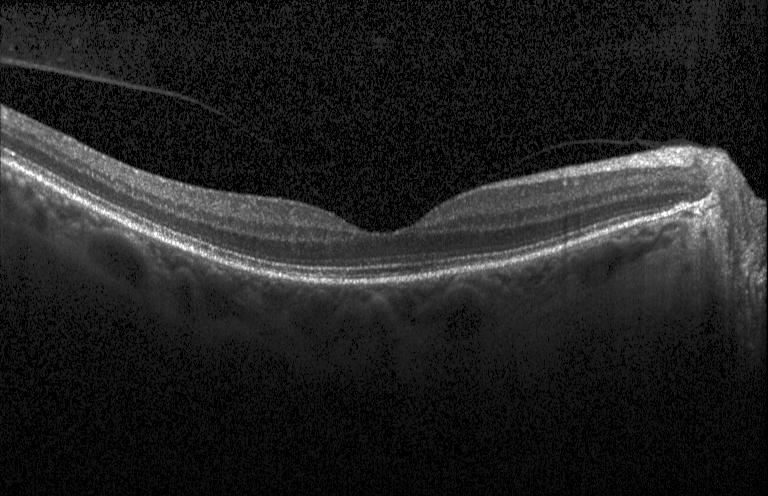
Finding: neither choroidal neovascularization, diabetic macular edema, nor drusen.